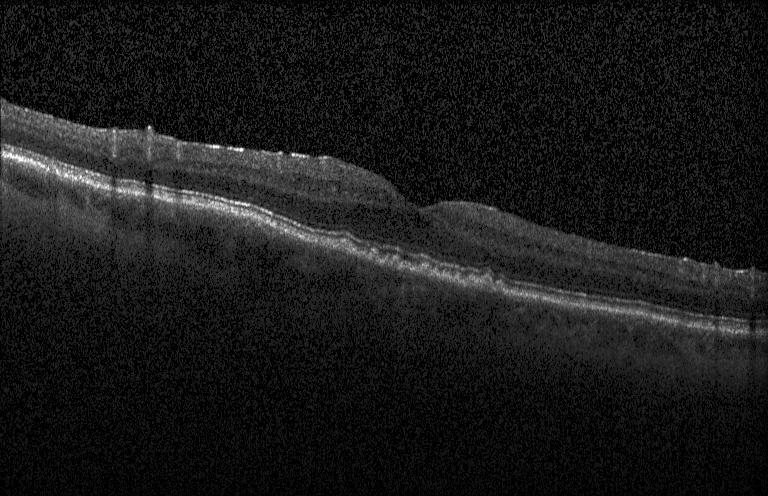 Through the macula · retinal OCT B-scan
Assessment: sub-RPE drusenoid deposits.